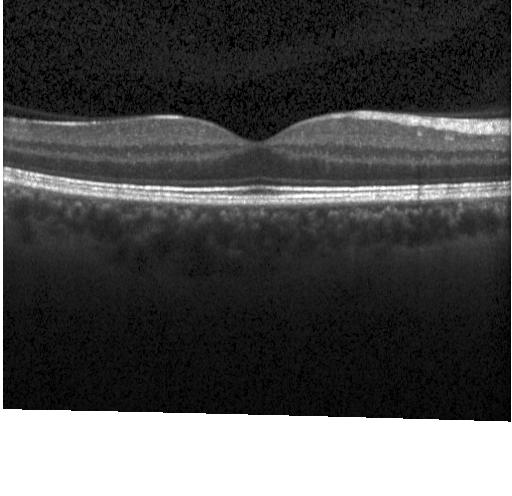

Optical coherence tomography B-scan — This B-scan demonstrates no CNV, DME, or drusen.